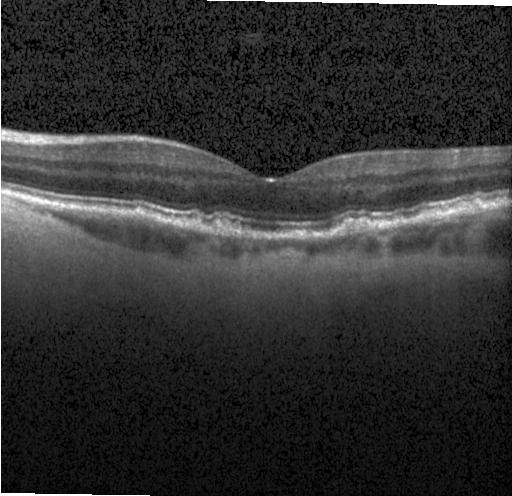
OCT line scan.
Macular OCT: sub-RPE drusenoid deposits.